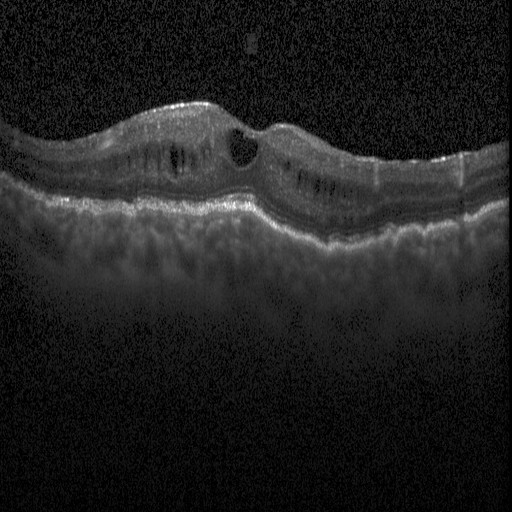
OCT B-scan; through the macula; spectral-domain OCT.
Dx: diabetic macular edema (DME).